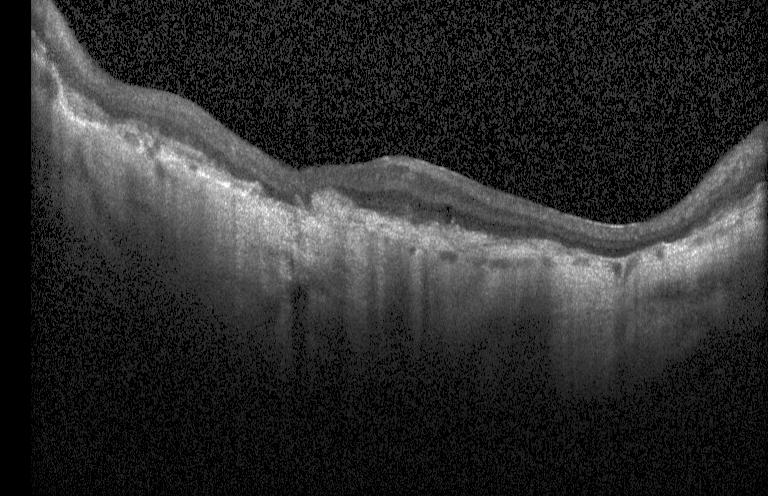

OCT B-scan
Impression: a choroidal neovascular membrane.